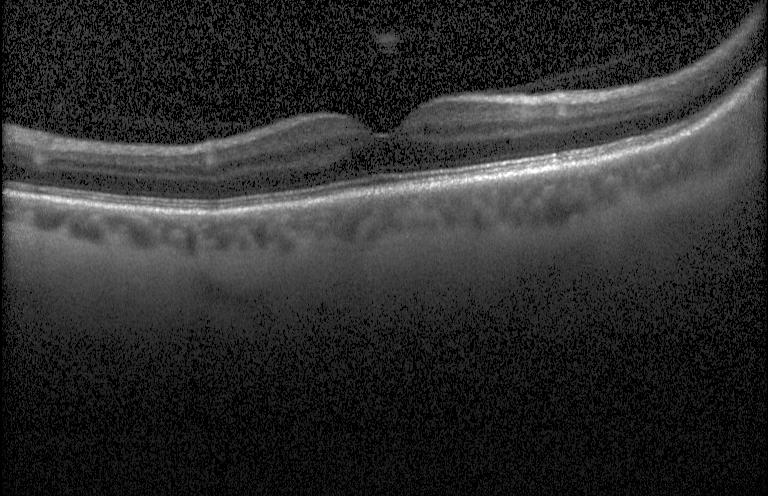 Finding: neither CNV, DME, nor drusen.